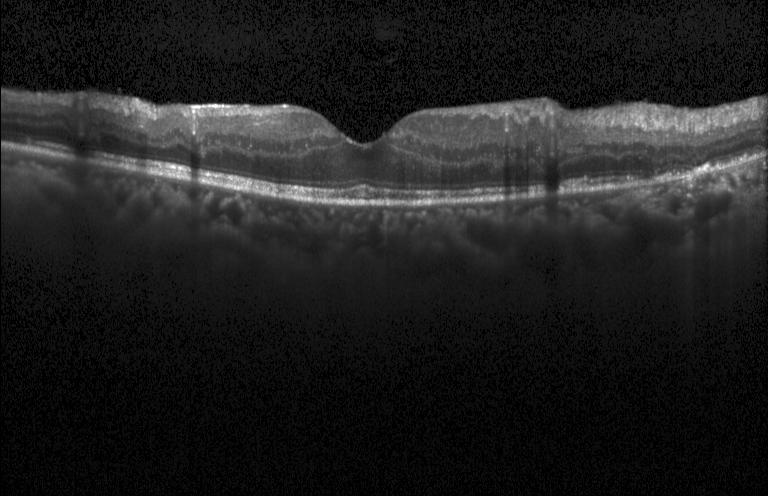

Centered on the fovea. Retinal OCT B-scan. Finding: diabetic macular edema.